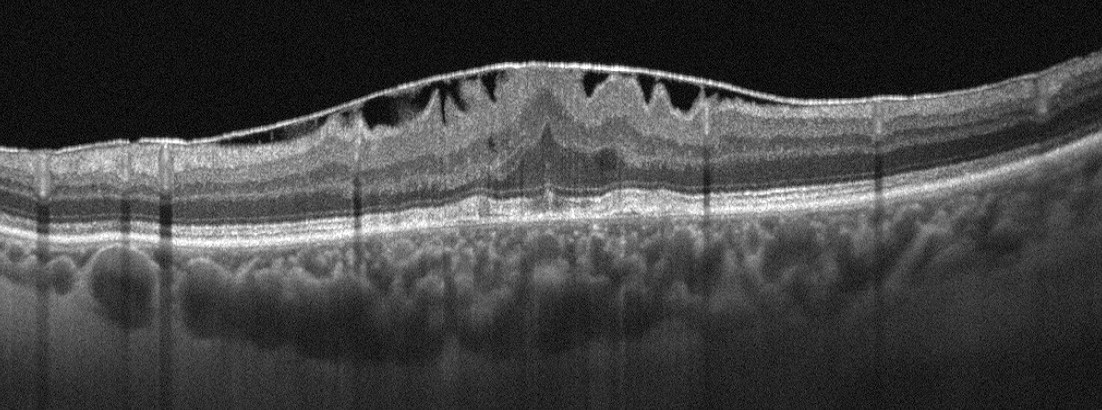 OCT B-scan
Finding: ERM.